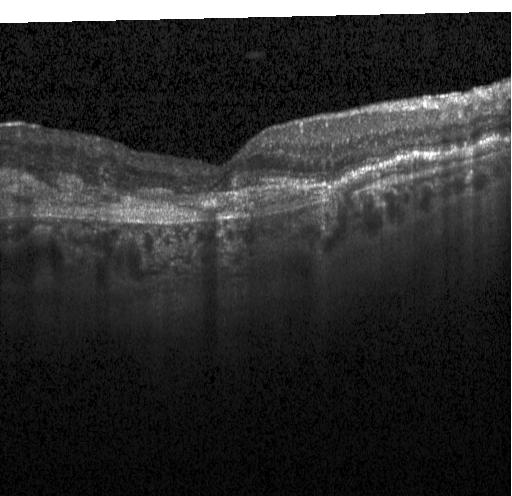 Impression: choroidal neovascularization (CNV).